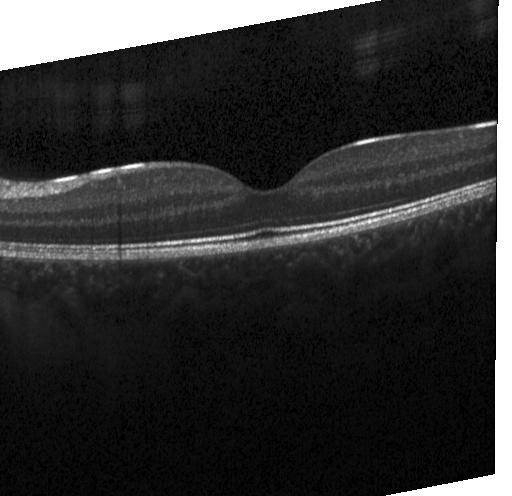 Diagnosis: neither CNV, DME, nor drusen.